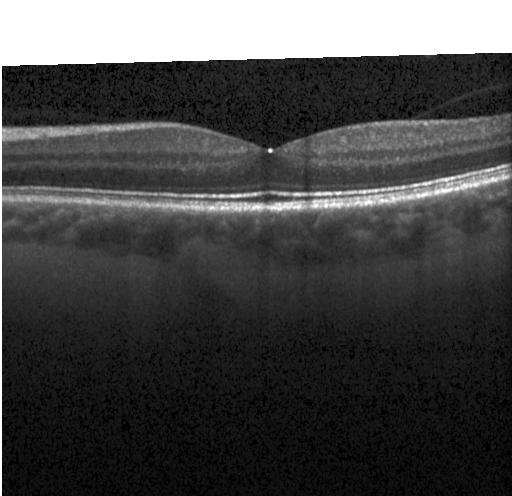 No CNV, DME, or drusen.